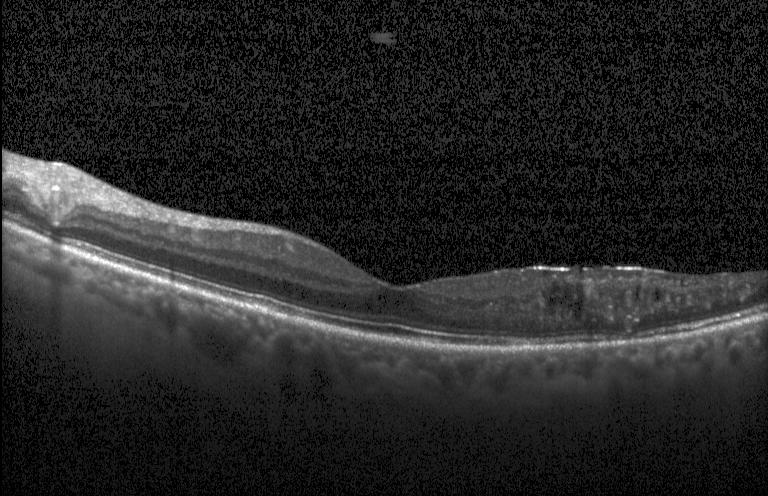

Retinal OCT B-scan · spectral-domain OCT.
Diabetic macular edema (DME).